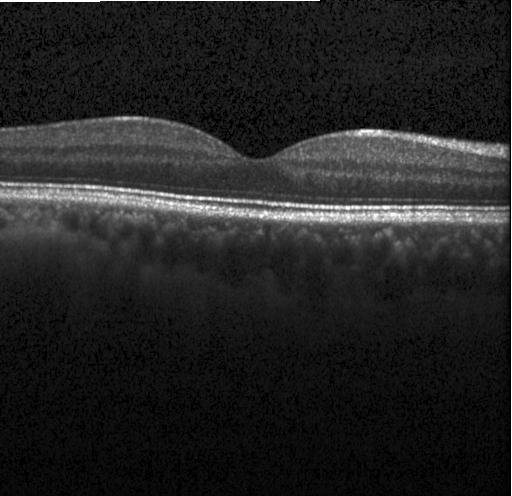

This B-scan demonstrates no CNV, DME, or drusen.